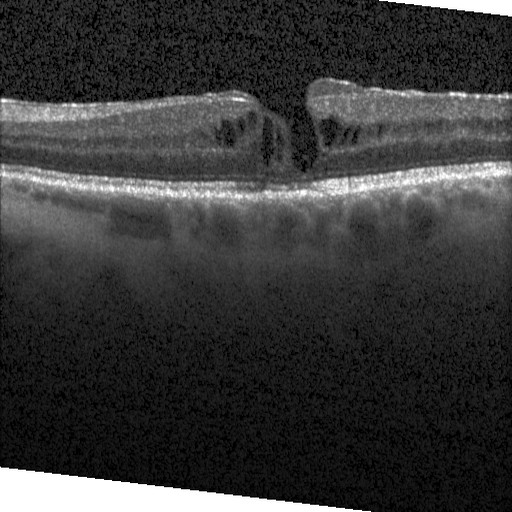

Impression: diabetic macular edema.